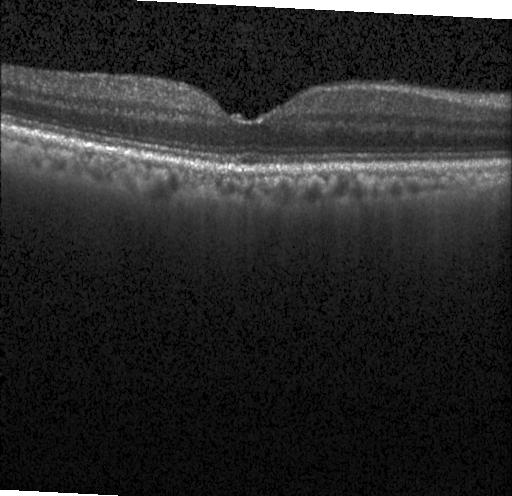

OCT B-scan · instrument: Heidelberg Spectralis — OCT finding: no CNV, no DME, and no drusen.